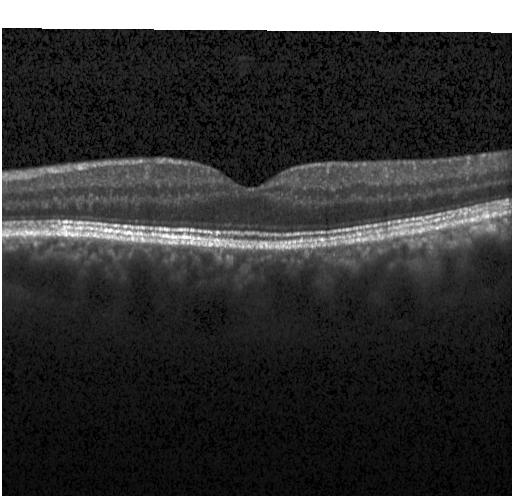
No evidence of CNV, DME, or drusen.